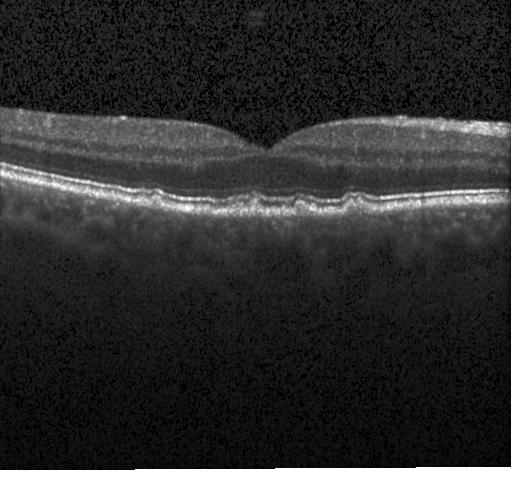
Optical coherence tomography scan. Instrument: Heidelberg Spectralis. Spectral-domain optical coherence tomography. Horizontal scan through the fovea.
This B-scan demonstrates multiple drusen.